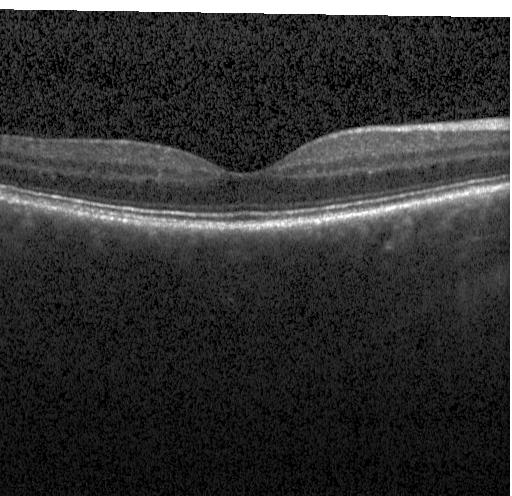
Impression: no evidence of choroidal neovascularization, diabetic macular edema, or drusen.